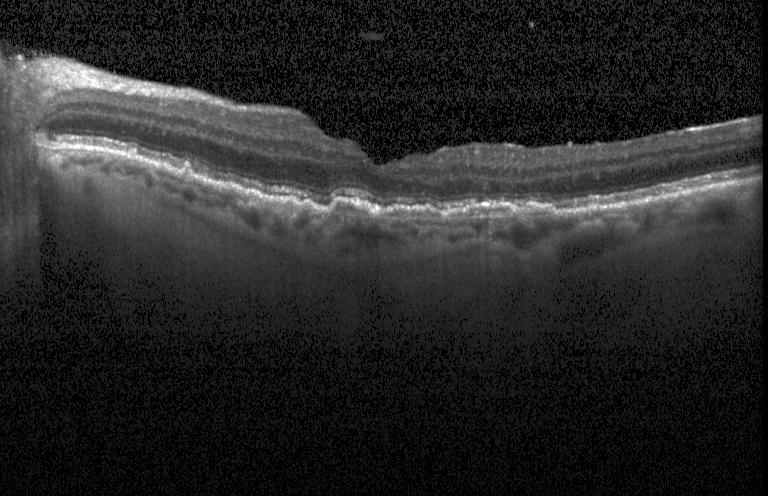

Assessment: drusen.